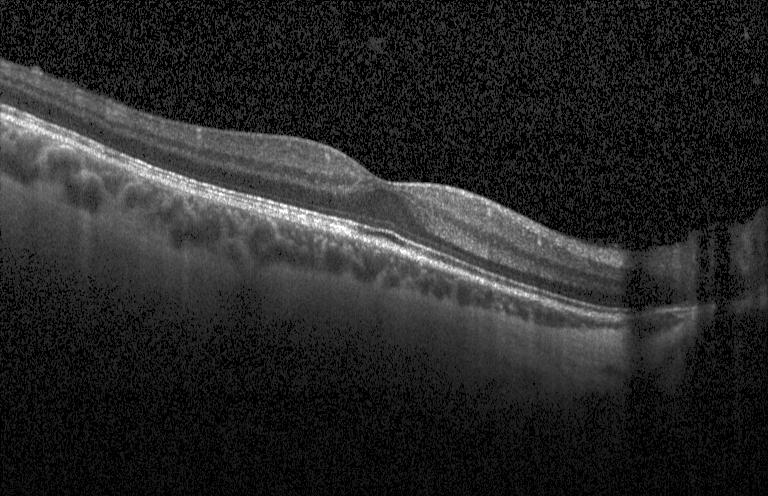 Retinal OCT cross-section showing no choroidal neovascularization, diabetic macular edema, or drusen.